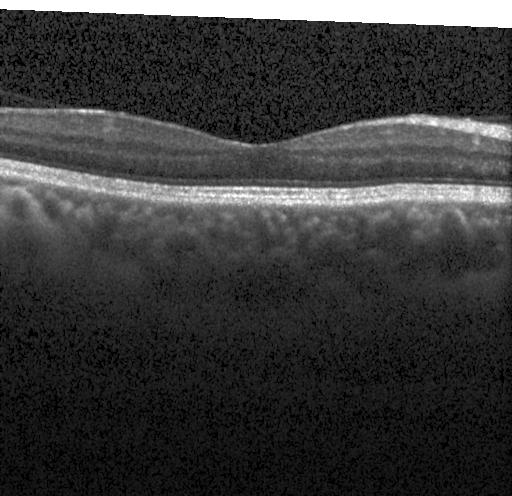

Optical coherence tomography B-scan — Macular OCT: neither choroidal neovascularization, diabetic macular edema, nor drusen.